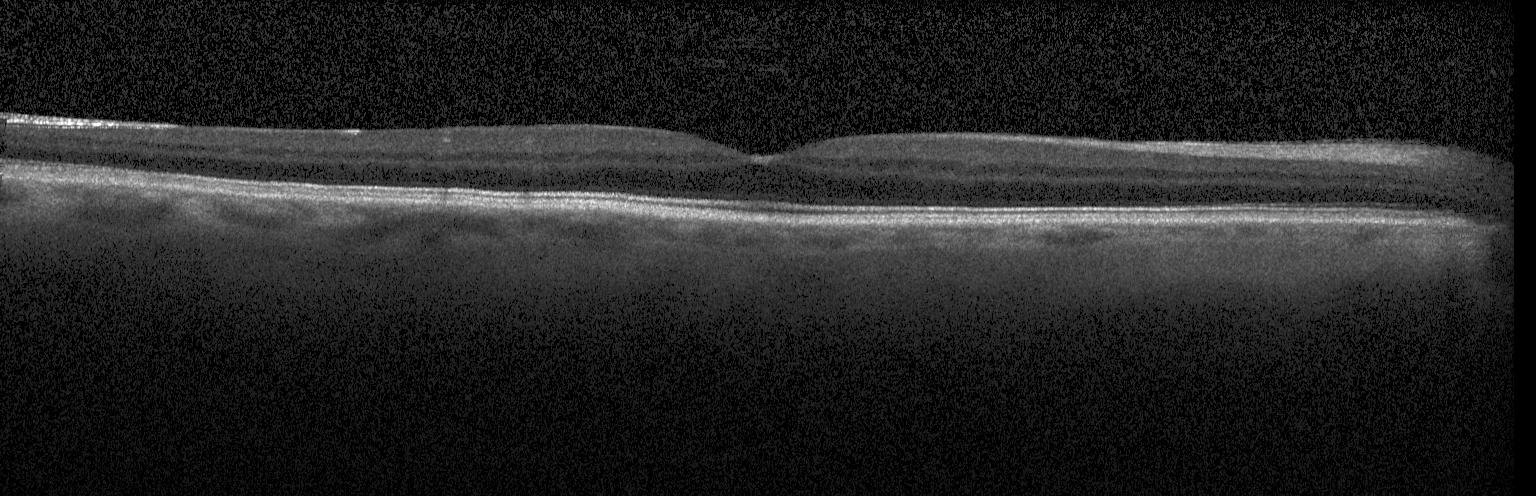

Heidelberg Spectralis, OCT B-scan, through the macula.
Assessment: neither choroidal neovascularization, diabetic macular edema, nor drusen.